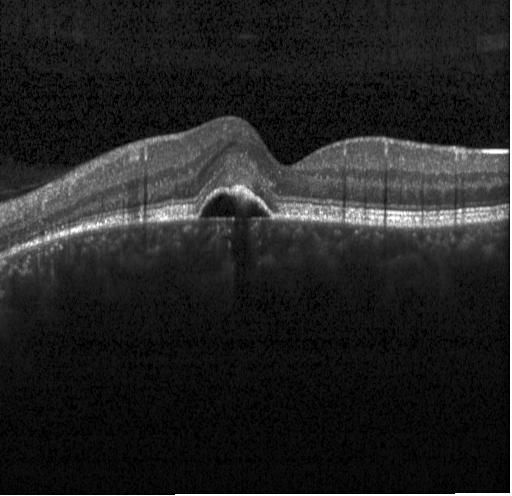

OCT line scan — Macular OCT: choroidal neovascularization.